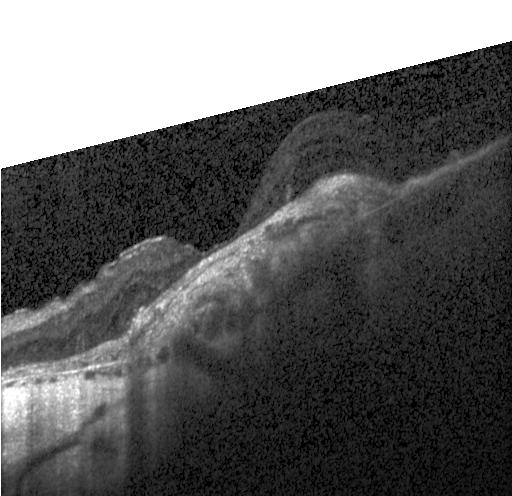

OCT B-scan
Finding: CNV.